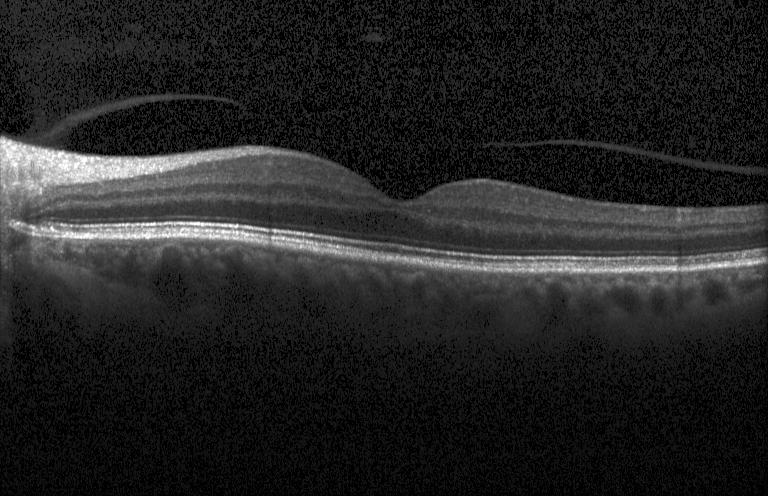

Heidelberg Spectralis OCT system; retinal OCT cross-section; macular scan.
No evidence of choroidal neovascularization, diabetic macular edema, or drusen.